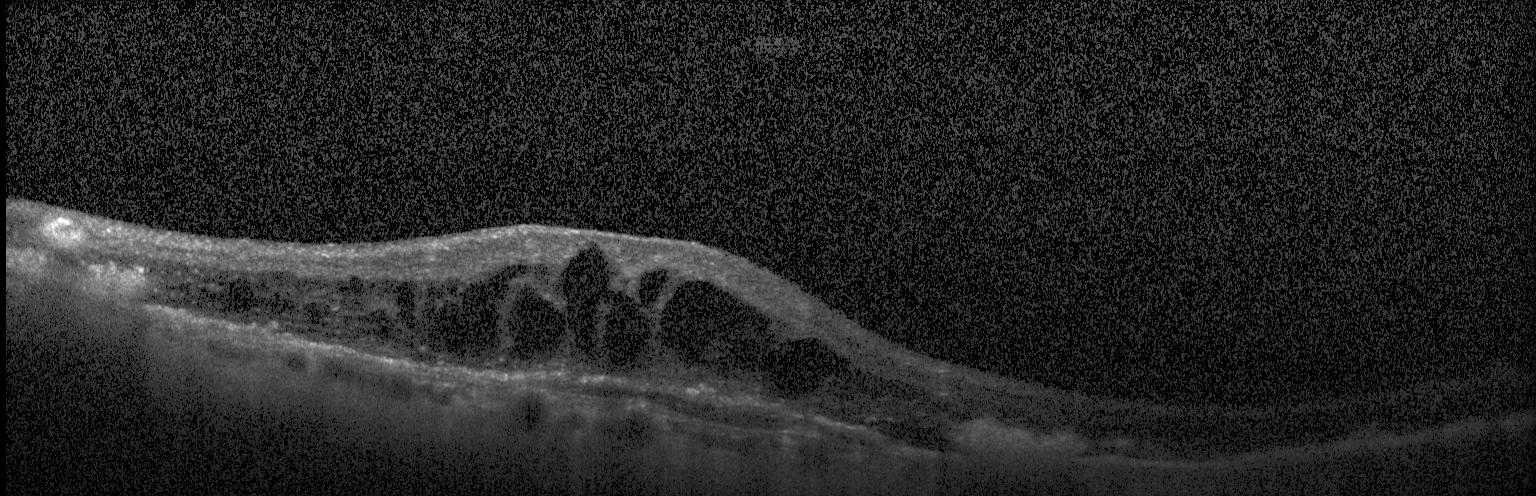

Optical coherence tomography B-scan — The scan shows choroidal neovascularization.